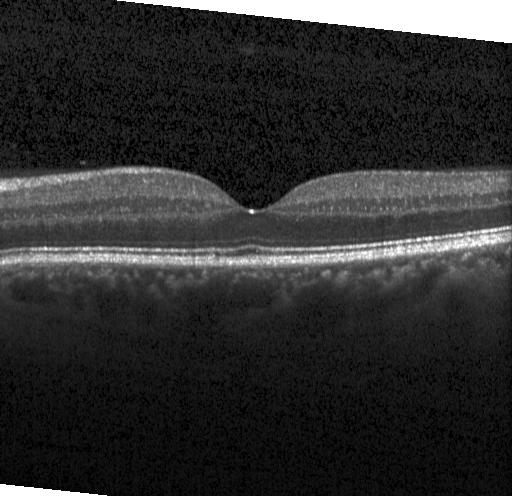
Impression: neither choroidal neovascularization, diabetic macular edema, nor drusen.